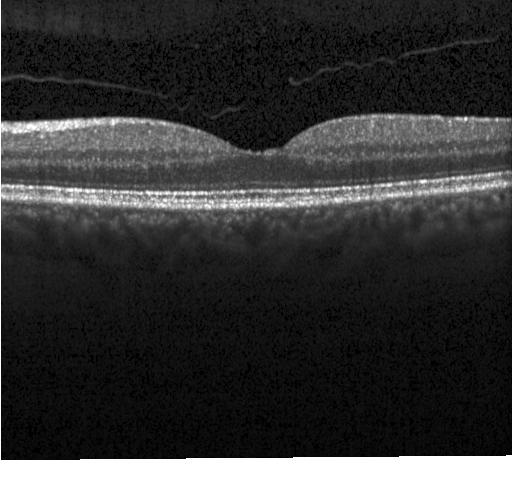
OCT B-scan · acquired on a Heidelberg Spectralis · macular scan
The scan shows no evidence of choroidal neovascularization, diabetic macular edema, or drusen.